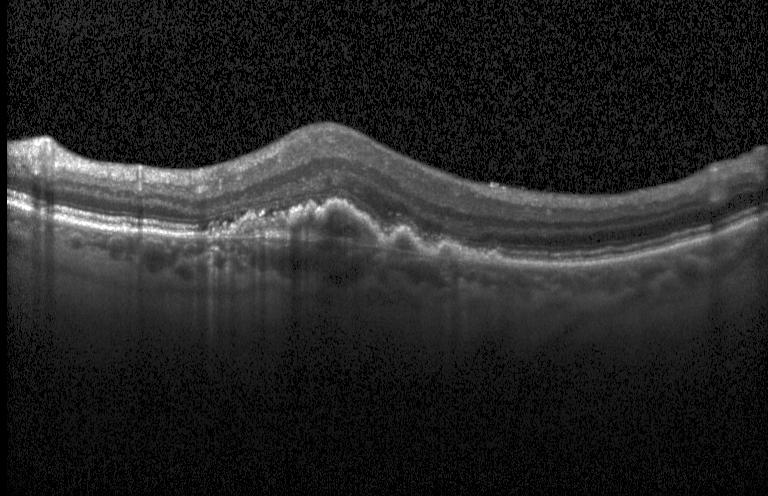 Optical coherence tomography B-scan — Diagnosis: a choroidal neovascular membrane.